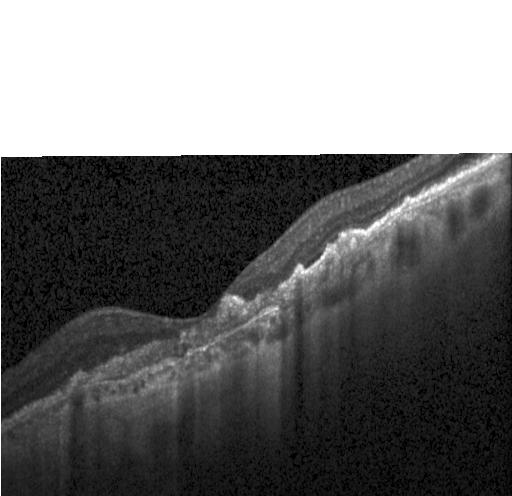
Optical coherence tomography B-scan.
Assessment: choroidal neovascularization.